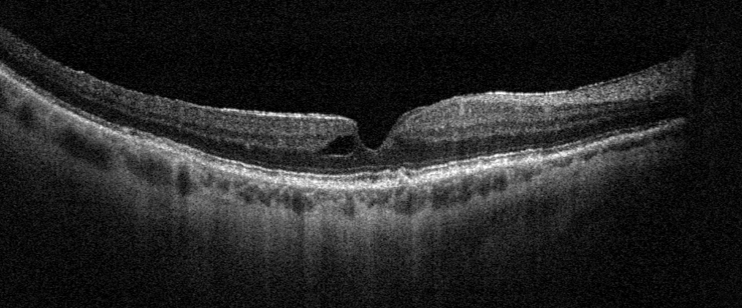

OCT B-scan; acquired on an Optovue Avanti RTVue XR. The scan shows vitreomacular interface disease.